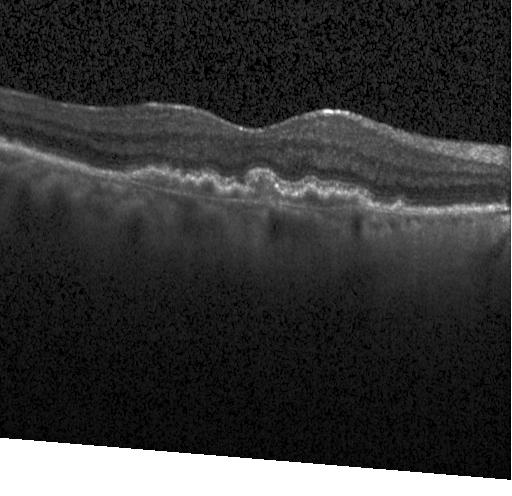

Impression: a choroidal neovascular membrane.